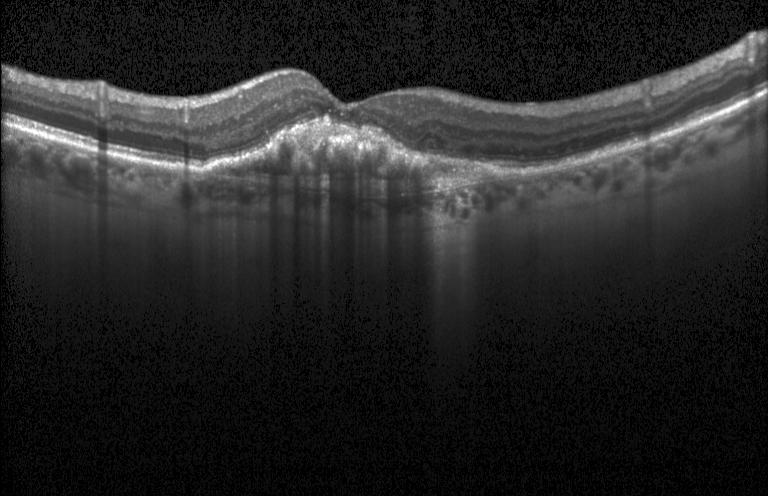 Spectral-domain OCT · optical coherence tomography scan.
Diagnosis: choroidal neovascularization.